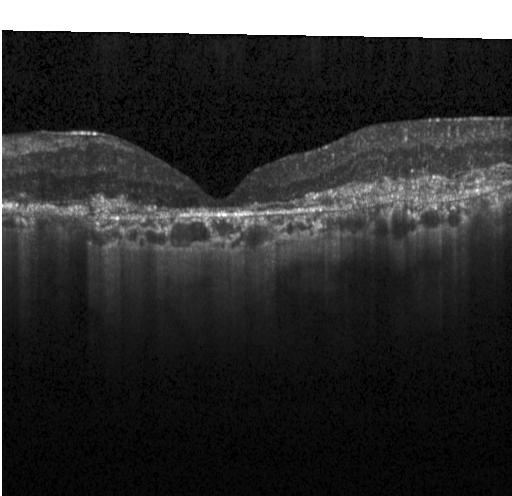
SD-OCT · horizontal scan through the fovea · instrument: Heidelberg Spectralis · retinal OCT cross-section
Diagnosis: a choroidal neovascular membrane.